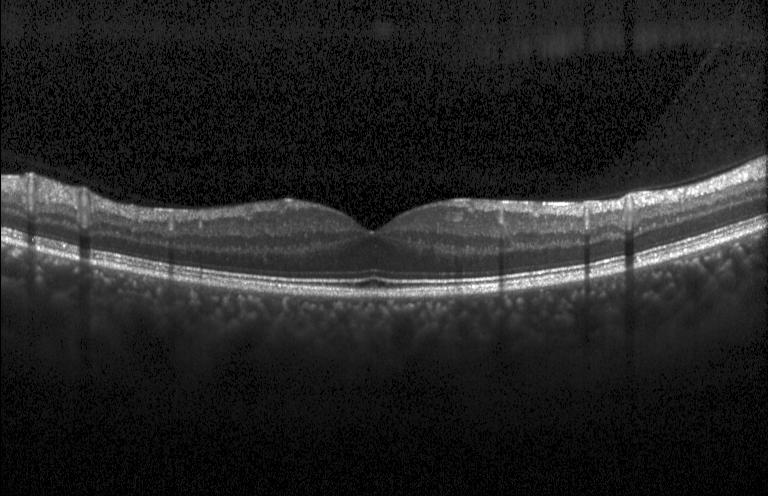 Instrument: Heidelberg Spectralis. Spectral-domain optical coherence tomography. Centered on the fovea. Retinal OCT B-scan. Finding: no choroidal neovascularization, no diabetic macular edema, and no drusen.